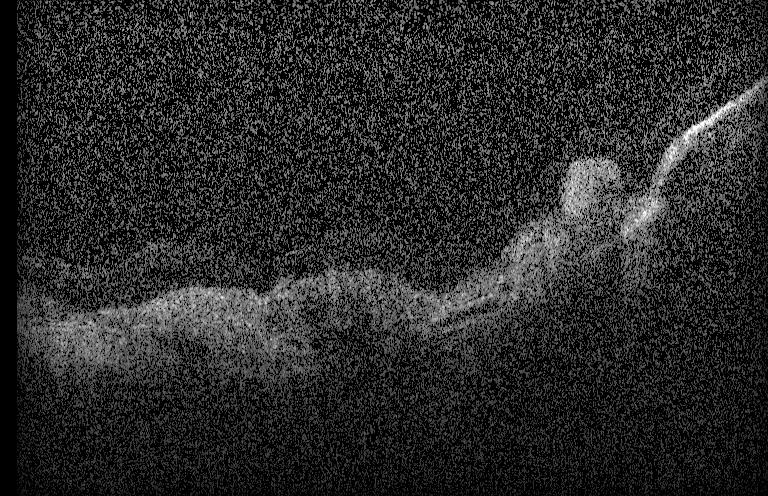
OCT B-scan.
Impression: a choroidal neovascular membrane.